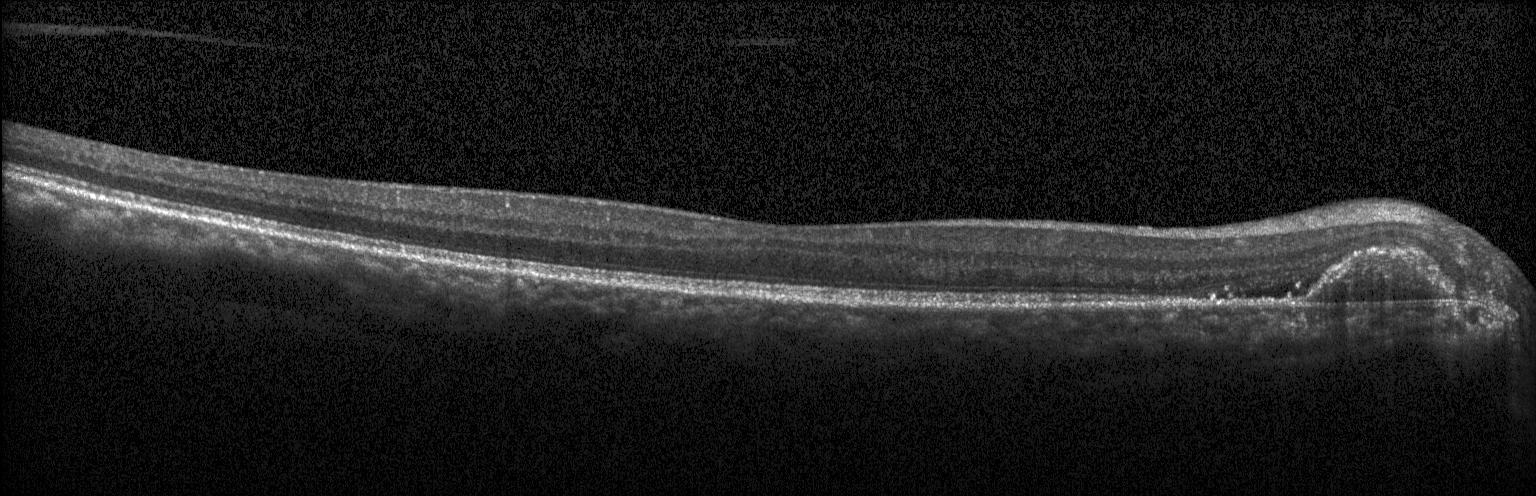 OCT line scan
Dx: choroidal neovascularization.